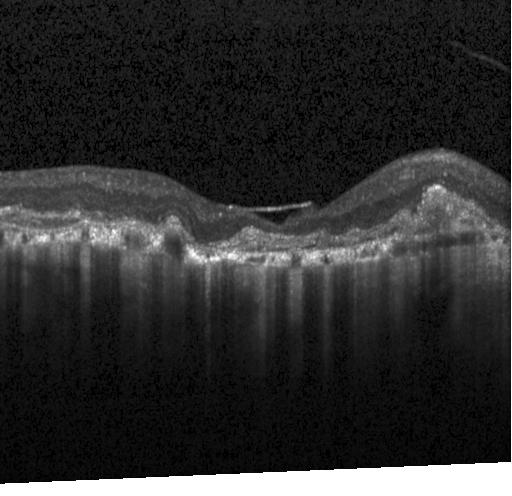 Finding: a choroidal neovascular membrane.